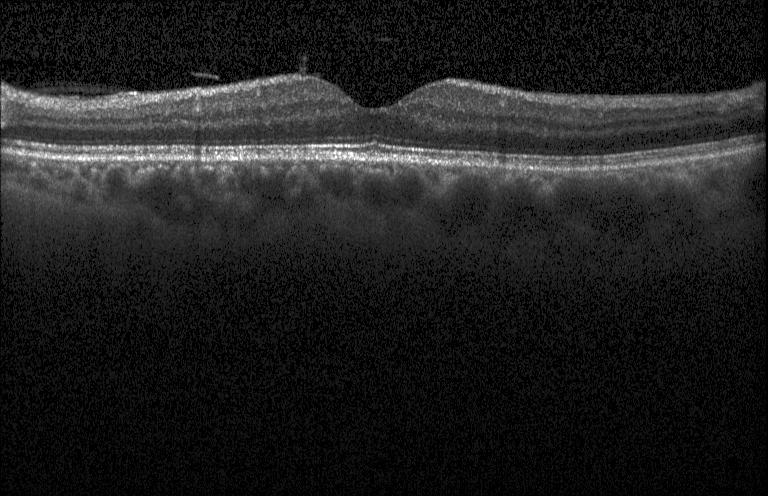
Retinal OCT cross-section, macular scan, Heidelberg Spectralis, SD-OCT — The scan shows no CNV, DME, or drusen.